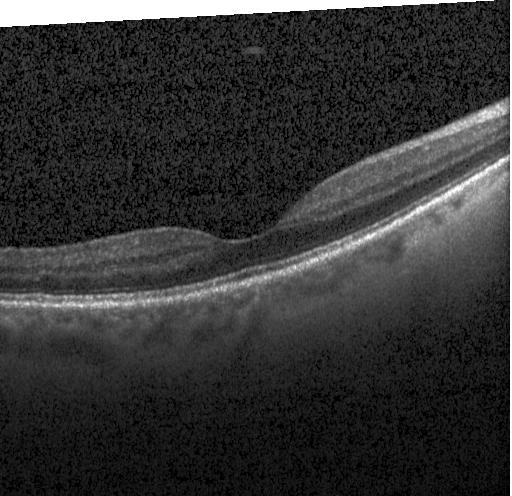

Instrument: Heidelberg Spectralis; retinal OCT B-scan; centered on the fovea; SD-OCT.
Diagnosis: neither CNV, DME, nor drusen.